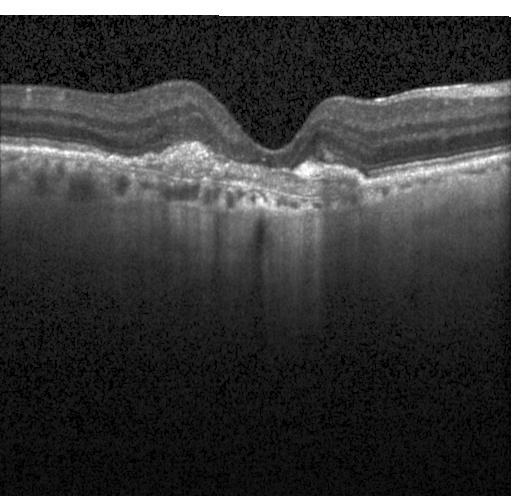 CNV.